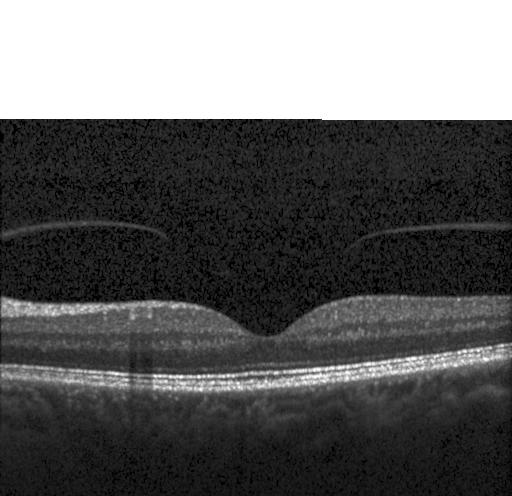 Finding: no evidence of choroidal neovascularization, diabetic macular edema, or drusen.